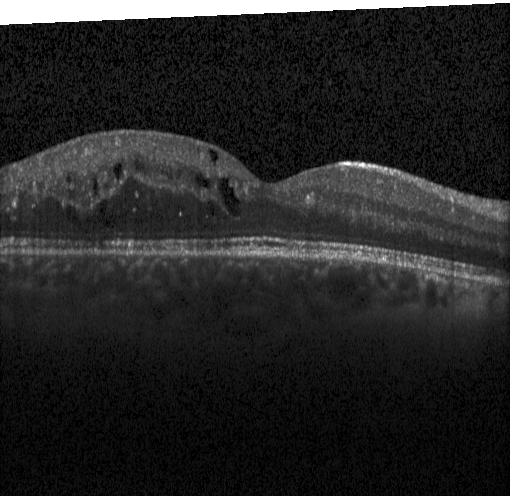
OCT line scan — Impression: diabetic macular edema (DME).